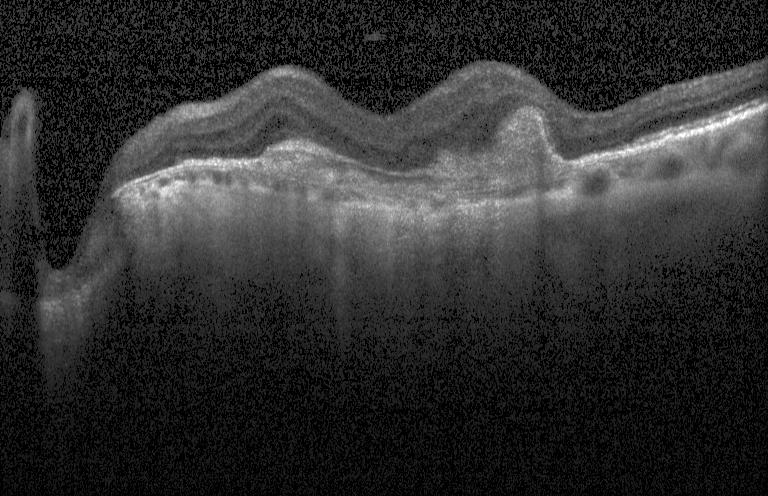

Finding: choroidal neovascularization.